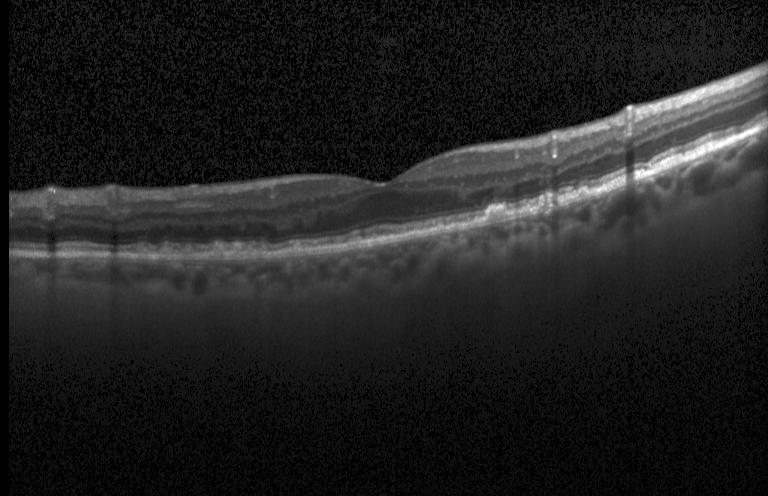 Centered on the fovea. Heidelberg Spectralis OCT system. Optical coherence tomography scan.
Diagnosis: sub-RPE drusenoid deposits.